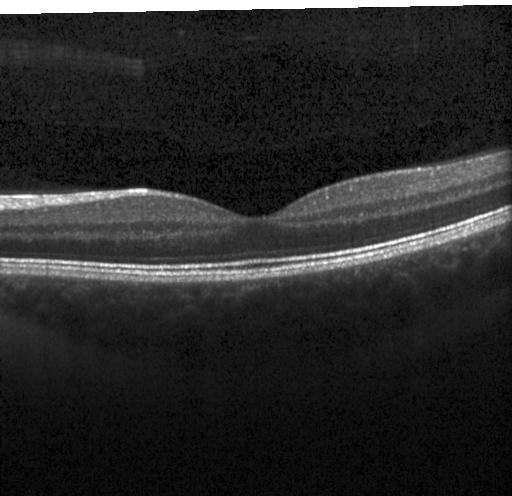
Spectral-domain optical coherence tomography. Retinal OCT B-scan. Acquired on a Heidelberg Spectralis.
OCT finding: no choroidal neovascularization, no diabetic macular edema, and no drusen.